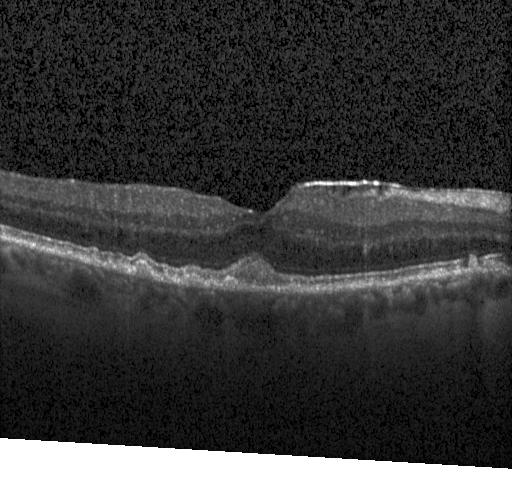

SD-OCT · retinal OCT B-scan · Heidelberg Spectralis OCT system — Impression: drusen.